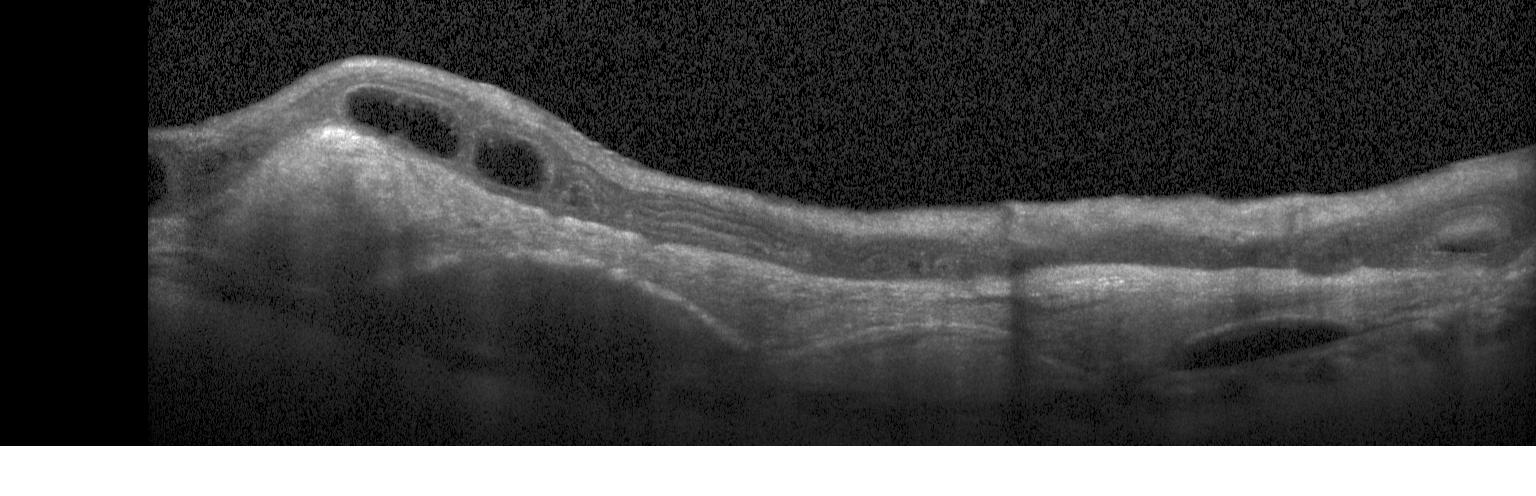 Spectral-domain OCT · through the macula · retinal OCT cross-section · instrument: Heidelberg Spectralis
Impression: choroidal neovascularization (CNV).